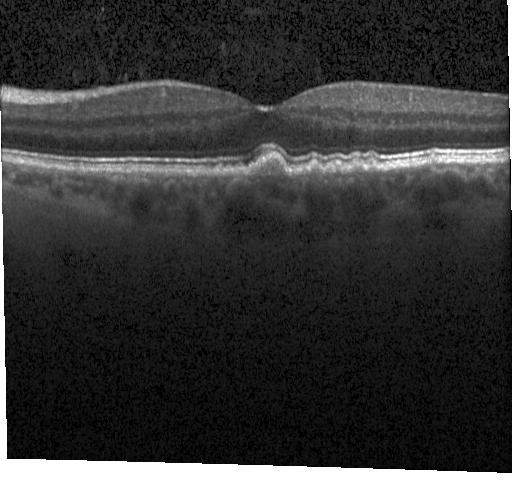
Finding: multiple drusen.